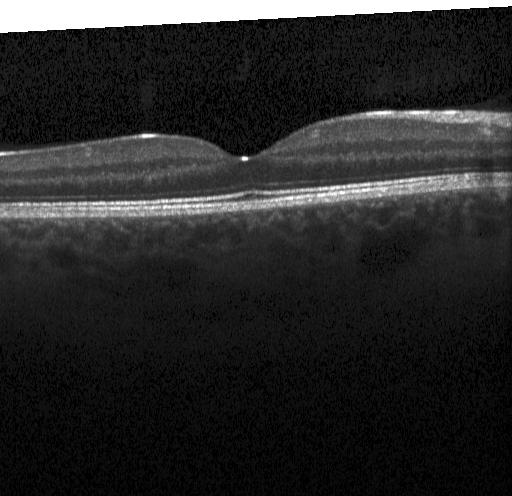

Centered on the fovea. Heidelberg Spectralis. OCT B-scan. Spectral-domain OCT. Dx: no CNV, no DME, and no drusen.